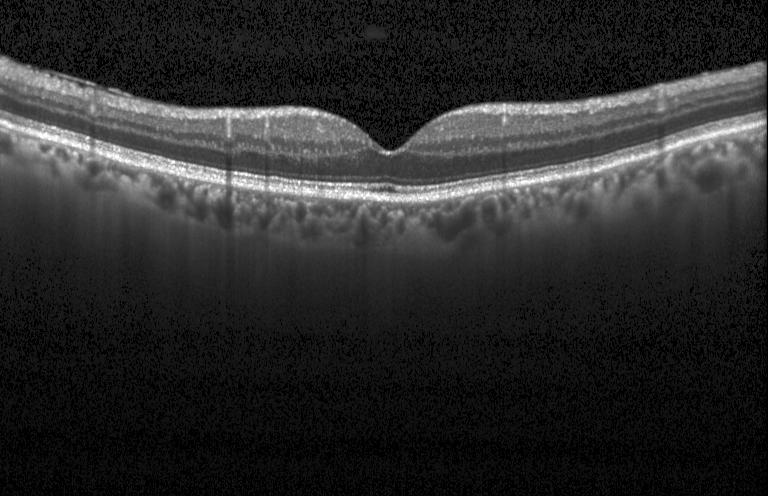
Optical coherence tomography B-scan, acquired on a Heidelberg Spectralis, spectral-domain OCT.
Assessment: neither choroidal neovascularization, diabetic macular edema, nor drusen.